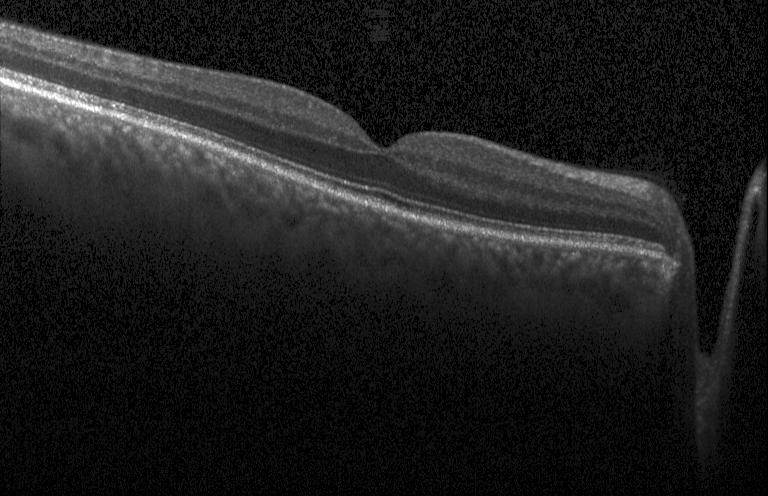

This B-scan demonstrates no CNV, no DME, and no drusen.